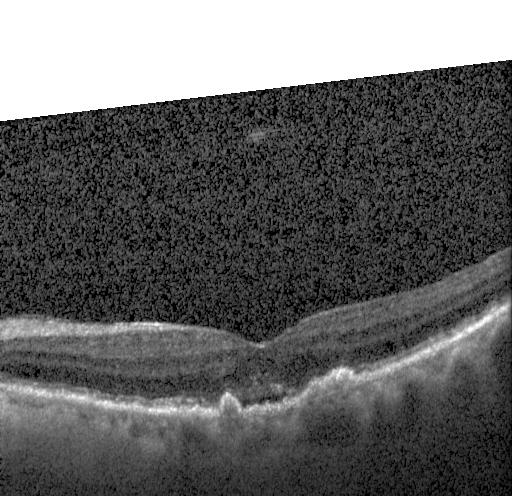

Heidelberg Spectralis · fovea-centered · OCT B-scan · SD-OCT. Diagnosis: a choroidal neovascular membrane.